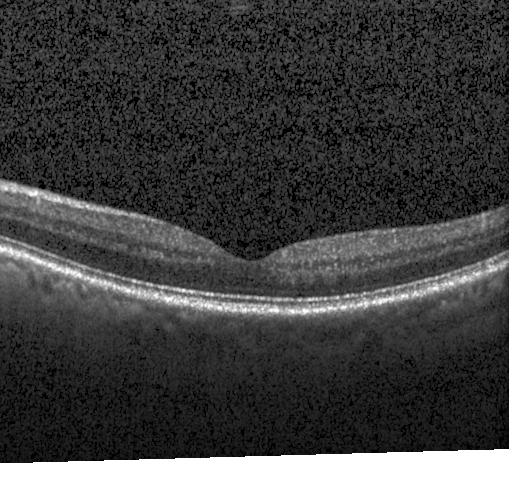

OCT B-scan — Diagnosis: neither CNV, DME, nor drusen.